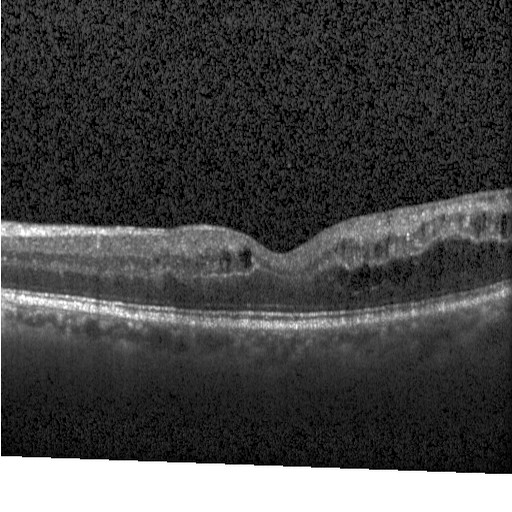

Retinal OCT cross-section; SD-OCT; horizontal scan through the fovea. This B-scan demonstrates DME.